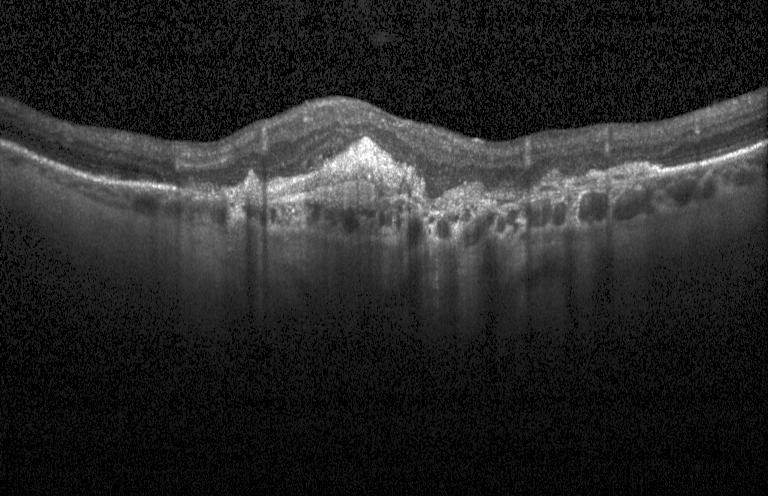
Spectral-domain OCT, OCT B-scan, Heidelberg Spectralis, centered on the fovea. Finding: a choroidal neovascular membrane.